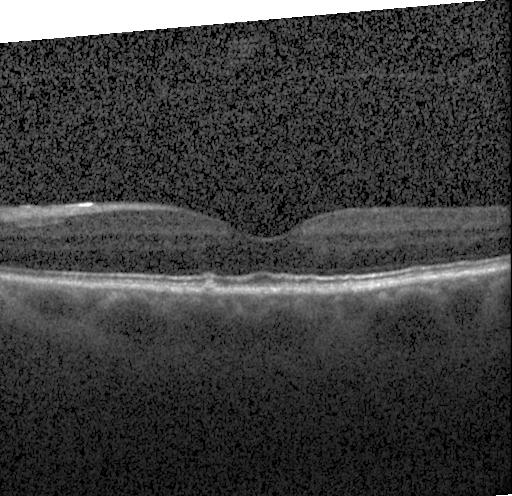
OCT B-scan. Impression: multiple drusen.